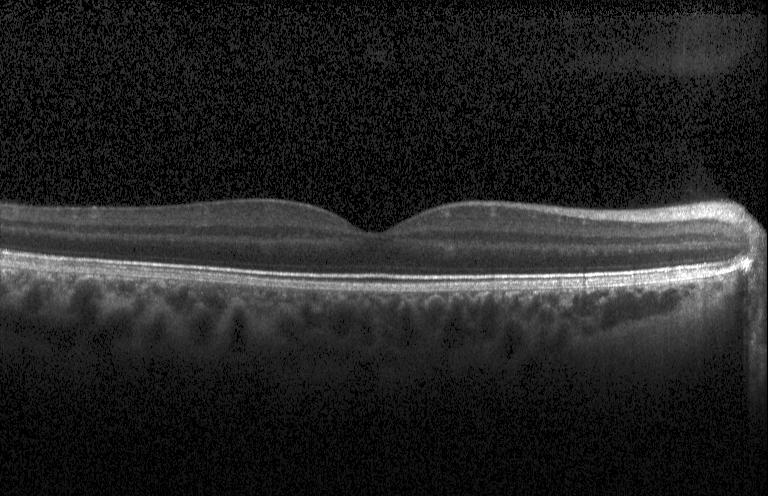

Dx: no evidence of choroidal neovascularization, diabetic macular edema, or drusen.